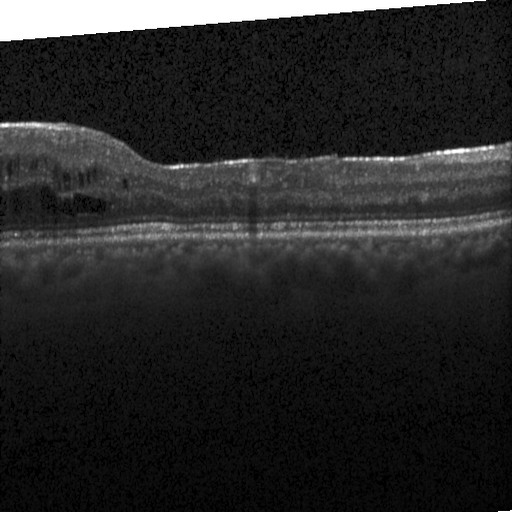
Retinal OCT cross-section showing diabetic macular edema.